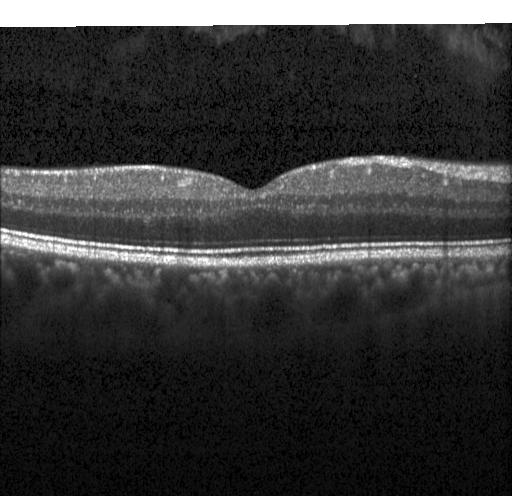
Retinal OCT B-scan. Acquired on a Heidelberg Spectralis. Spectral-domain OCT. Assessment: no evidence of choroidal neovascularization, diabetic macular edema, or drusen.